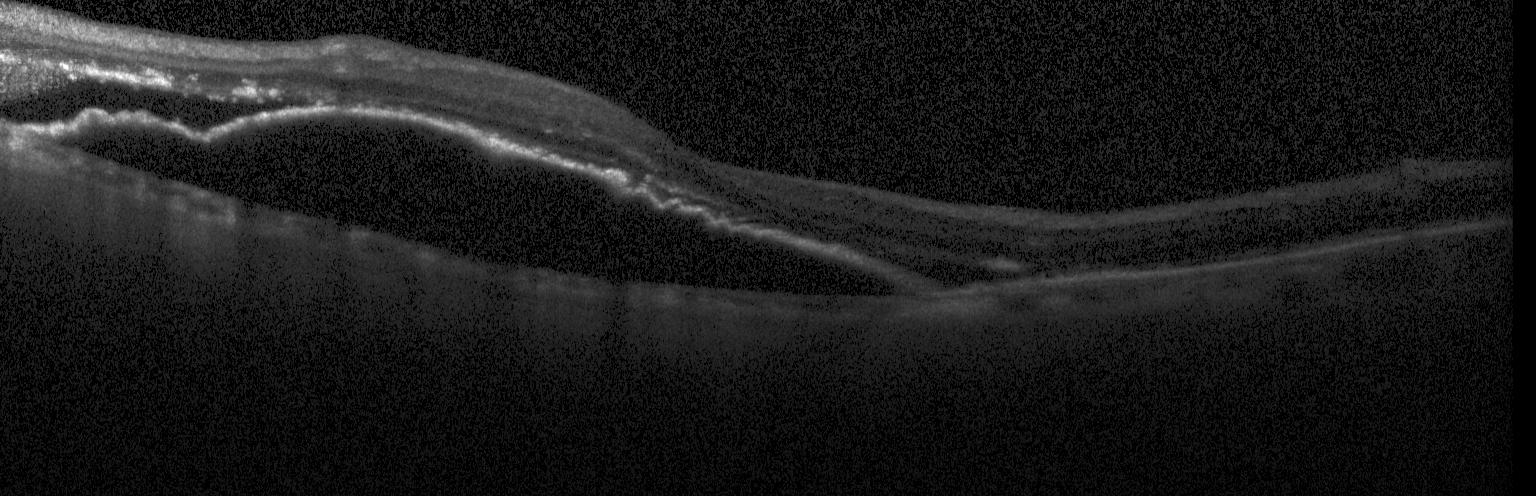

OCT line scan · Heidelberg Spectralis OCT system — Finding: choroidal neovascularization.